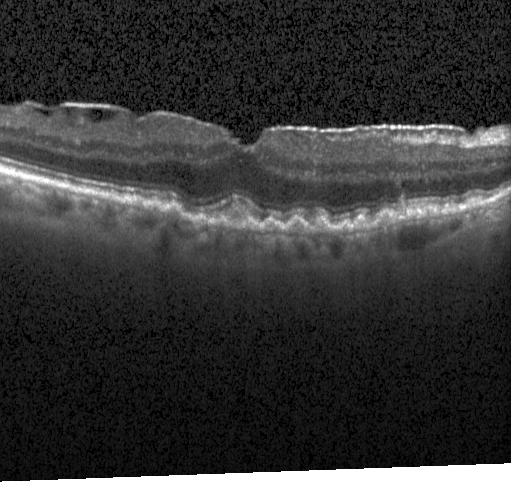

Spectral-domain optical coherence tomography · optical coherence tomography B-scan · Heidelberg Spectralis OCT system
Impression: drusen.